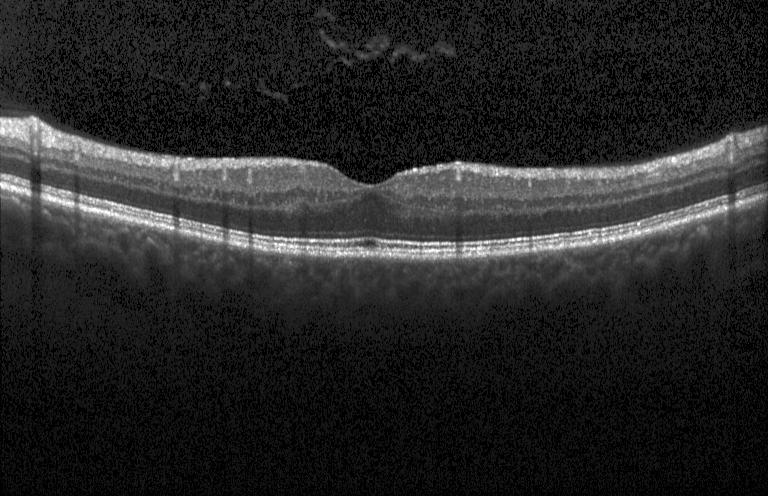

Retinal OCT B-scan. Diagnosis: no CNV, no DME, and no drusen.